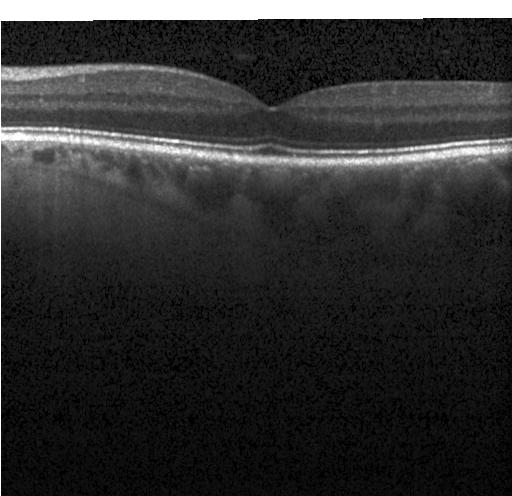

Spectral-domain OCT B-scan: neither CNV, DME, nor drusen.